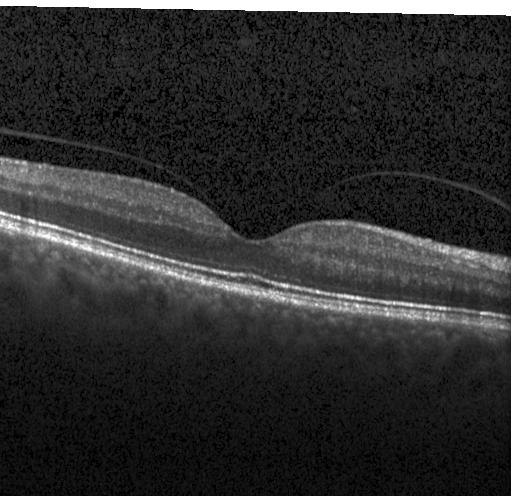
Horizontal scan through the fovea; optical coherence tomography B-scan; spectral-domain optical coherence tomography — The scan shows no choroidal neovascularization, diabetic macular edema, or drusen.